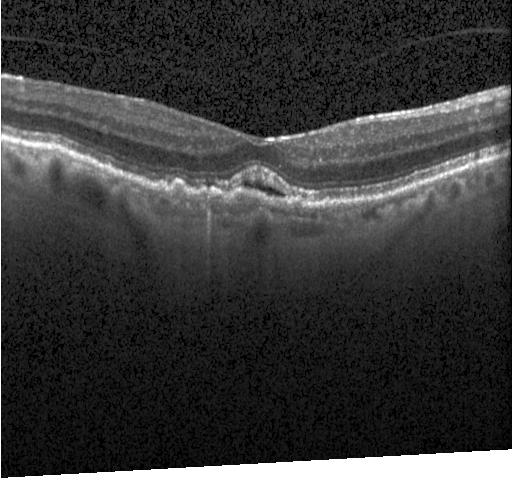
Assessment: CNV.